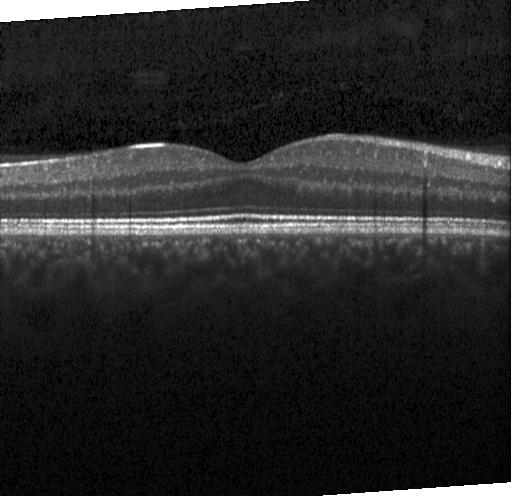
Fovea-centered, retinal OCT B-scan, Heidelberg Spectralis — Finding: no CNV, no DME, and no drusen.